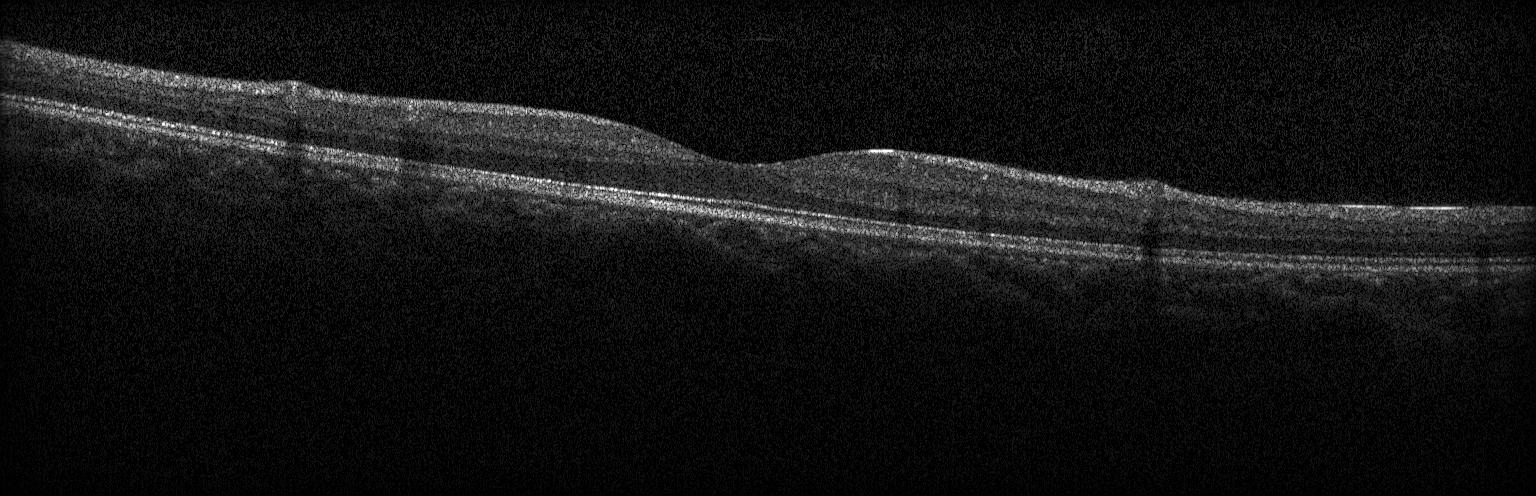 This B-scan demonstrates no evidence of choroidal neovascularization, diabetic macular edema, or drusen.